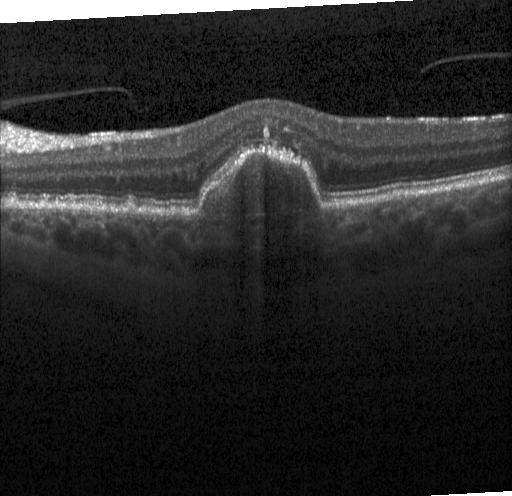 Assessment: CNV.